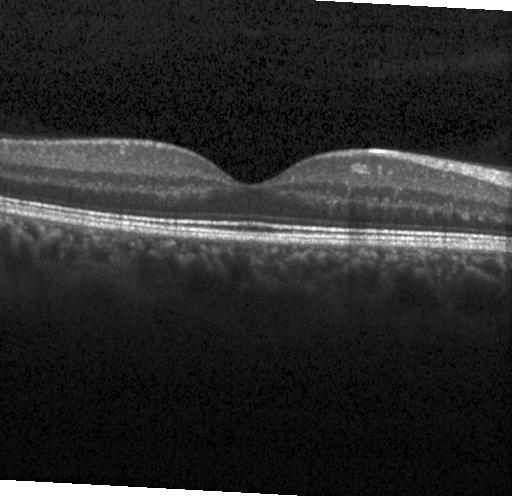

Retinal OCT cross-section.
Finding: no evidence of CNV, DME, or drusen.